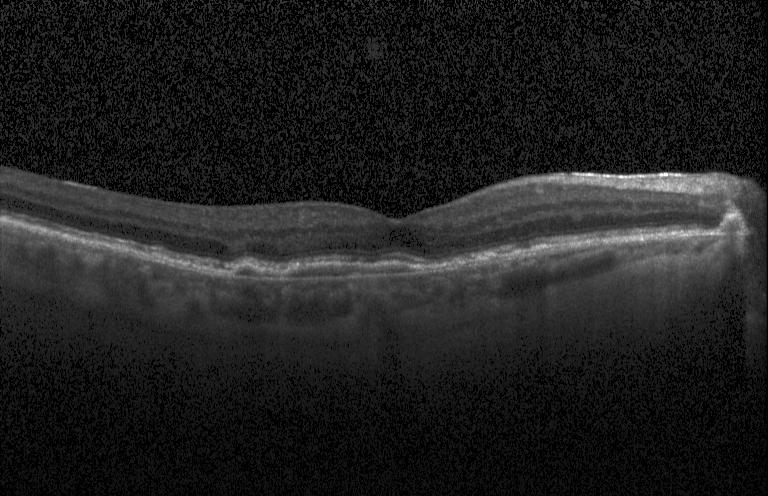
Impression: choroidal neovascularization.